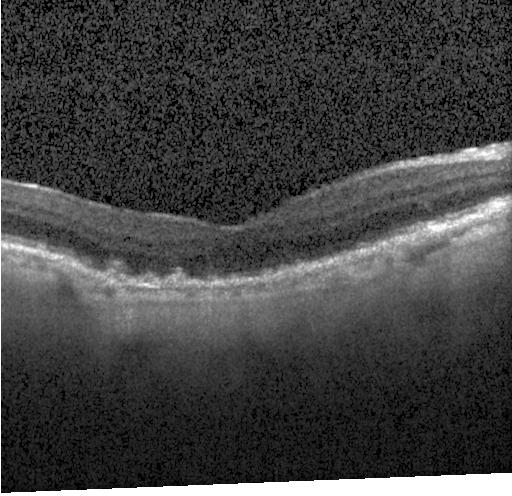
Retinal OCT B-scan. Impression: choroidal neovascularization.